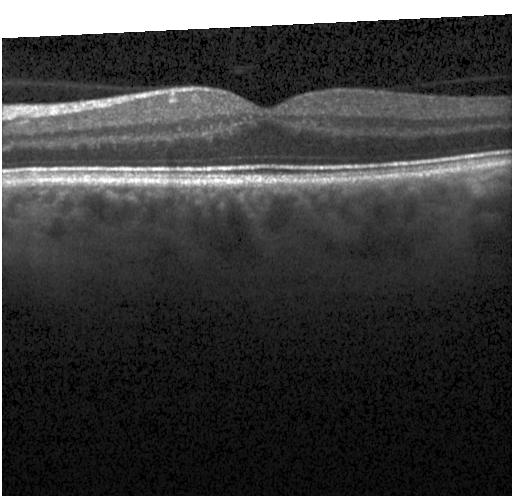
Spectral-domain OCT B-scan: neither choroidal neovascularization, diabetic macular edema, nor drusen.